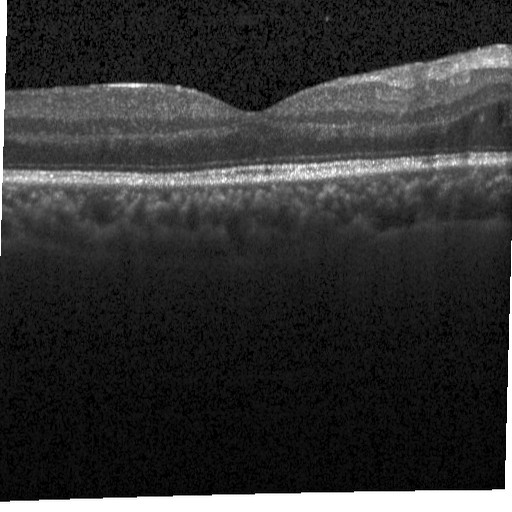 Finding: diabetic macular edema (DME).